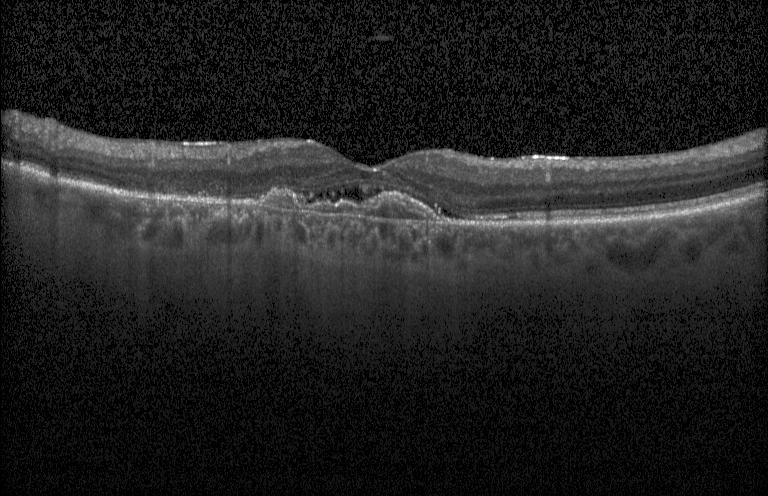 Horizontal scan through the fovea. Instrument: Heidelberg Spectralis. Retinal OCT B-scan. Spectral-domain OCT — This B-scan demonstrates choroidal neovascularization (CNV).